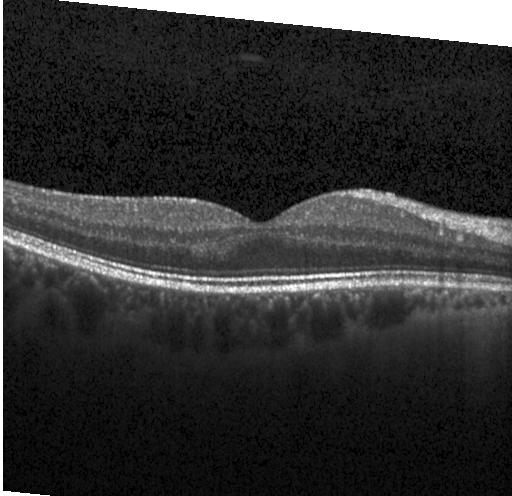 Spectral-domain OCT · optical coherence tomography scan · centered on the fovea
Dx: neither CNV, DME, nor drusen.